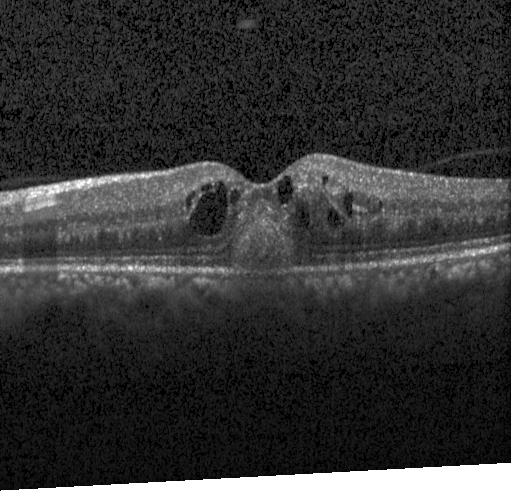
Retinal OCT B-scan, spectral-domain OCT, instrument: Heidelberg Spectralis.
Impression: choroidal neovascularization.